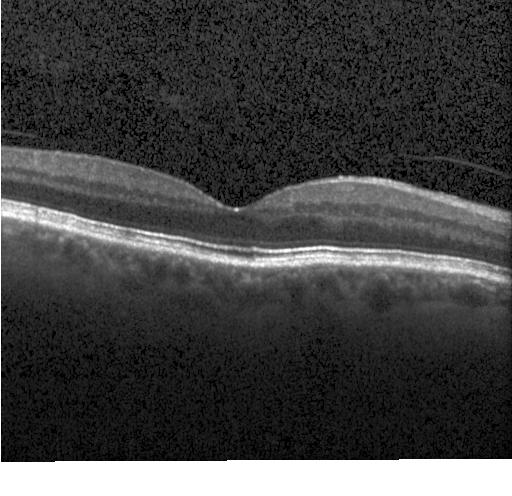
This B-scan demonstrates neither choroidal neovascularization, diabetic macular edema, nor drusen.